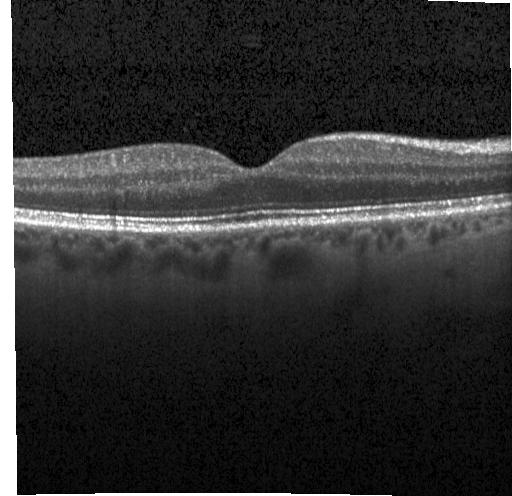
Finding: no choroidal neovascularization, diabetic macular edema, or drusen.